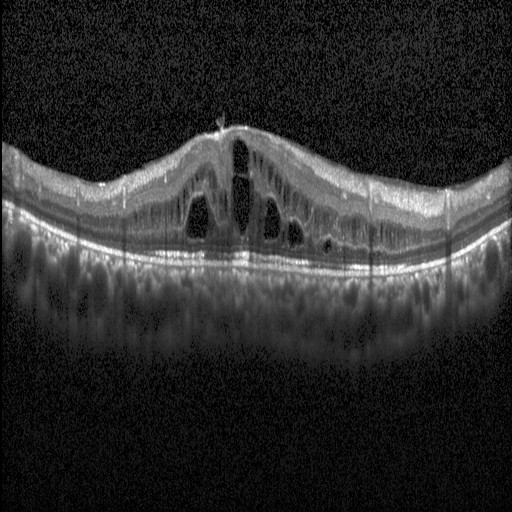
Instrument: Heidelberg Spectralis; spectral-domain optical coherence tomography; retinal OCT cross-section; macular scan. Diagnosis: DME.